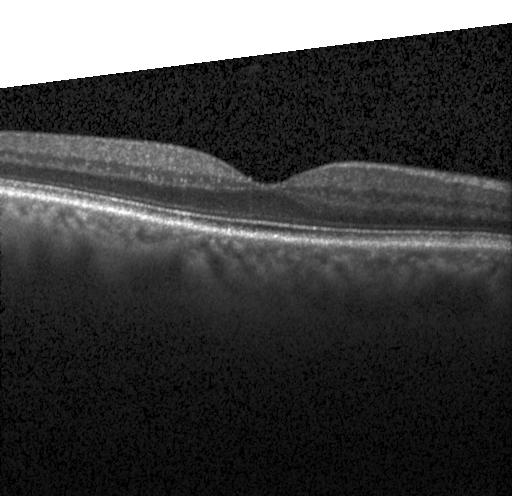

Diagnosis: no CNV, no DME, and no drusen.